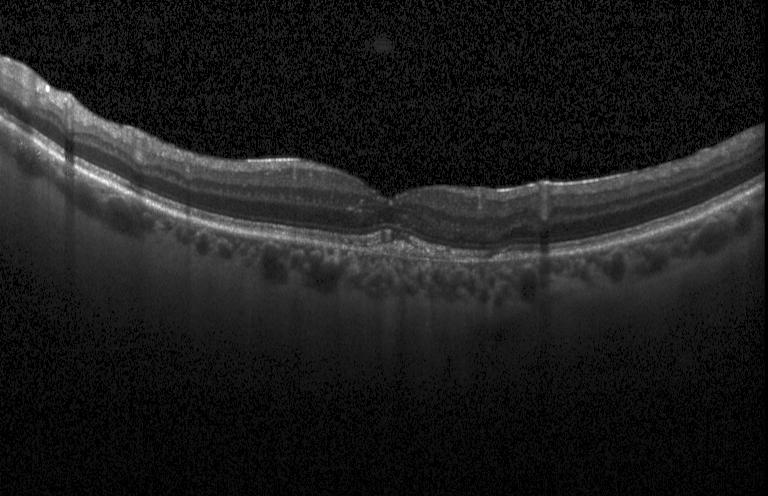
Retinal OCT B-scan. Heidelberg Spectralis. Assessment: a choroidal neovascular membrane.